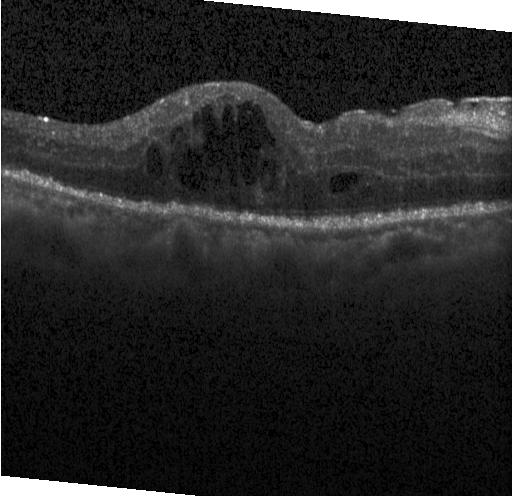

Diagnosis: diabetic macular edema.